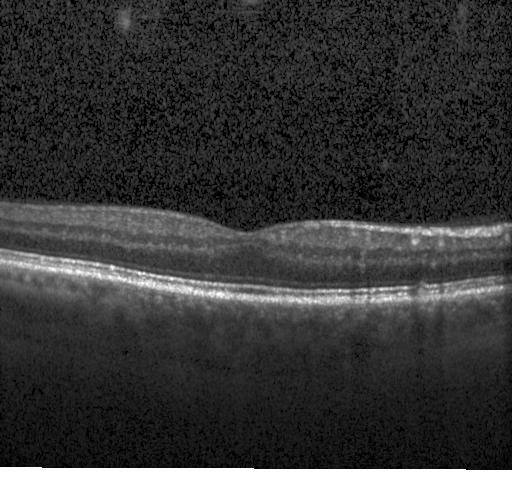

The scan shows no CNV, DME, or drusen.